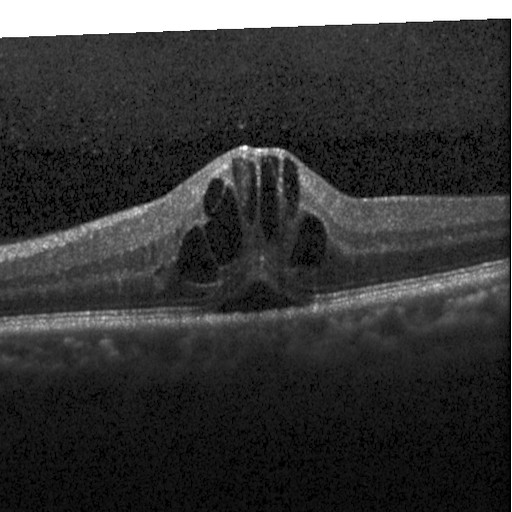

Impression: diabetic macular edema.